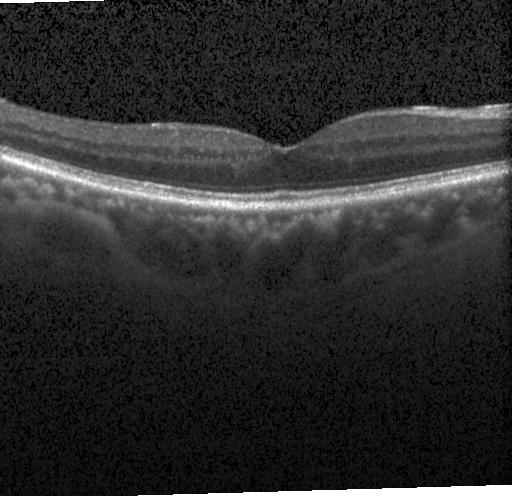

SD-OCT · optical coherence tomography B-scan · fovea-centered — Diagnosis: no choroidal neovascularization, no diabetic macular edema, and no drusen.